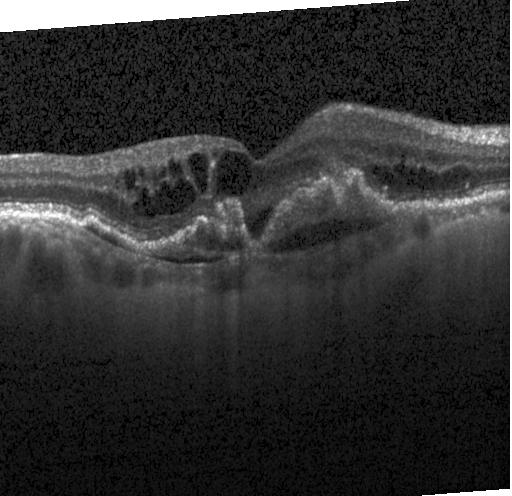 Impression: choroidal neovascularization.